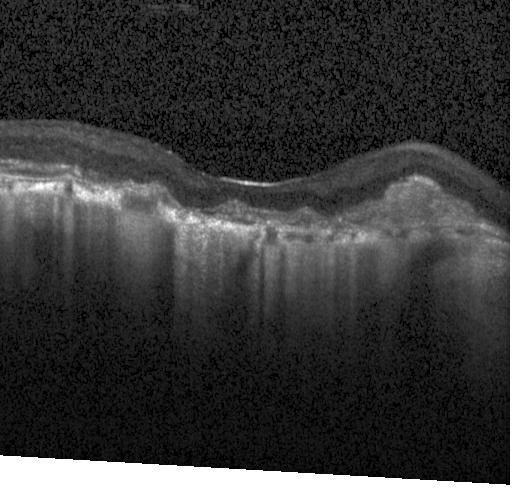
OCT B-scan. Through the macula. SD-OCT. CNV.